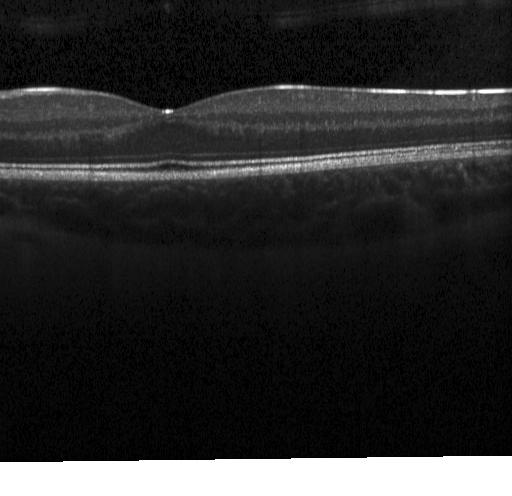
Diagnosis: neither choroidal neovascularization, diabetic macular edema, nor drusen.